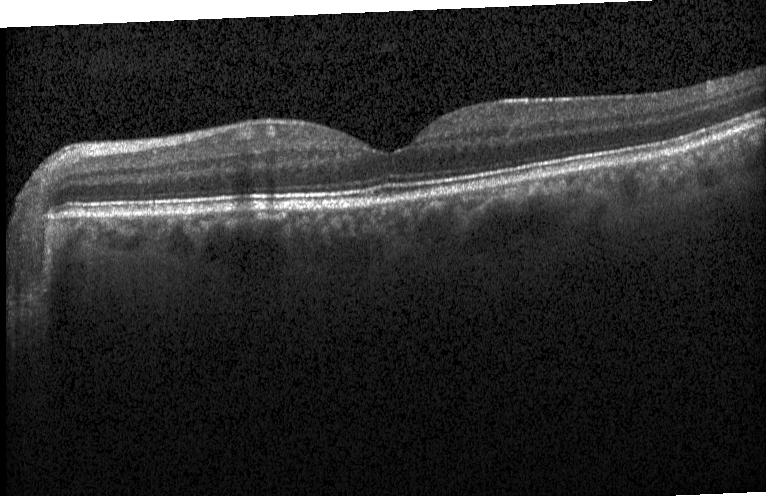 Optical coherence tomography B-scan. Through the macula. Instrument: Heidelberg Spectralis — Macular OCT: no choroidal neovascularization, diabetic macular edema, or drusen.